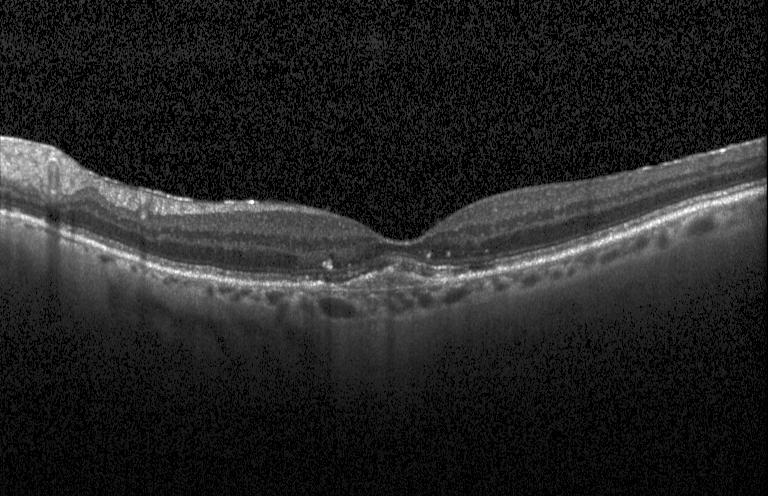

OCT finding: a choroidal neovascular membrane.